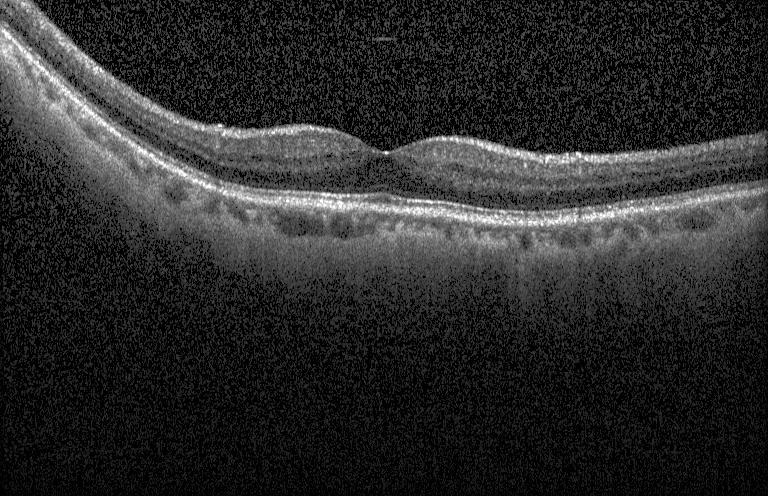
No evidence of choroidal neovascularization, diabetic macular edema, or drusen.